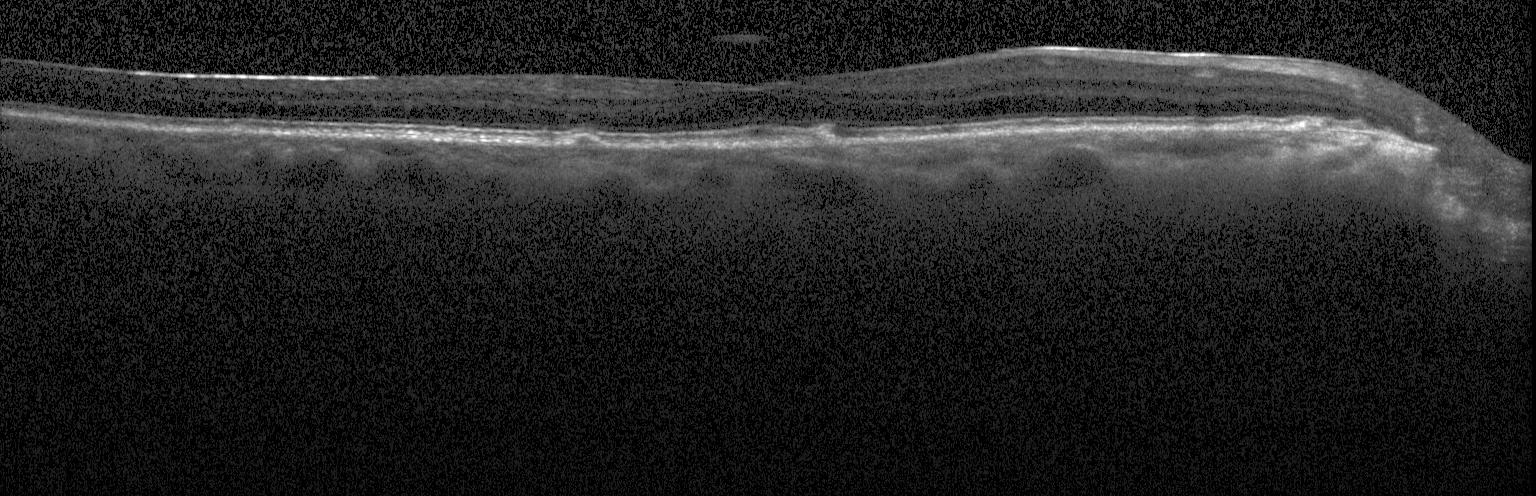
Retinal OCT cross-section. Assessment: sub-RPE drusenoid deposits.